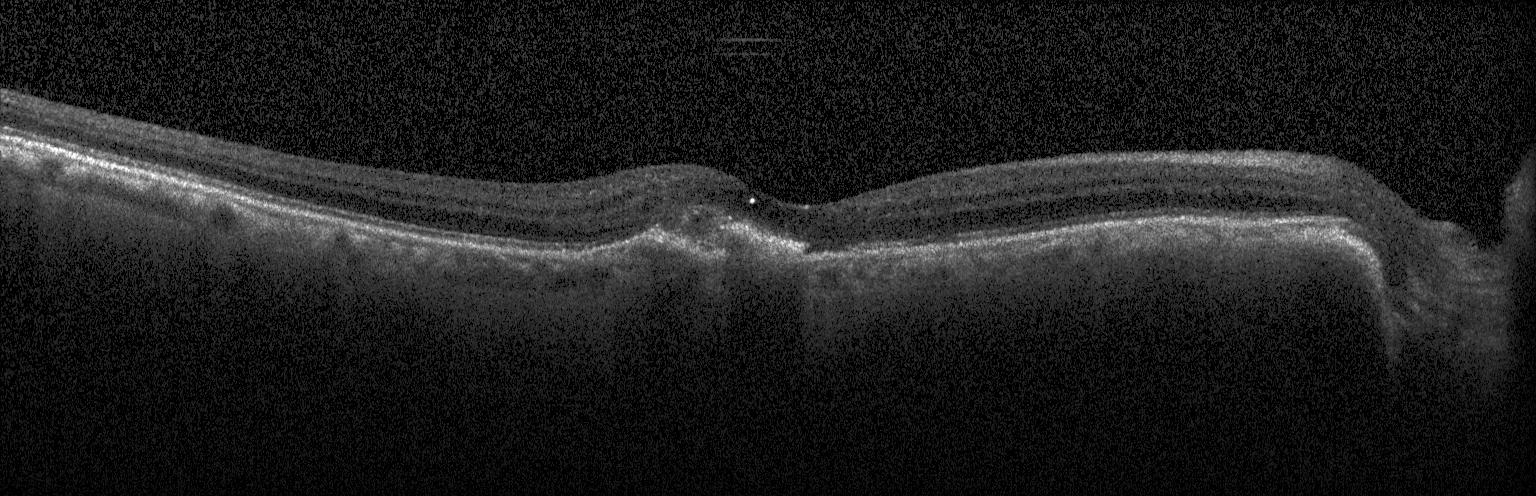
Instrument: Heidelberg Spectralis; macular scan; OCT B-scan; SD-OCT
OCT finding: choroidal neovascularization.